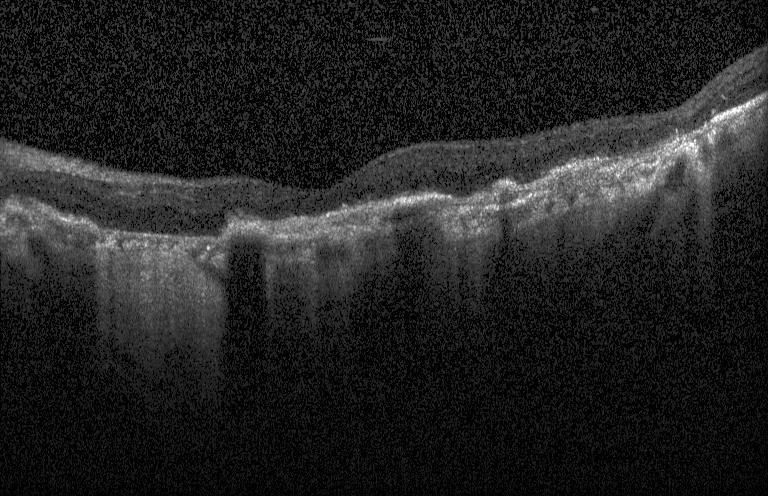

Macular scan · spectral-domain OCT · optical coherence tomography B-scan · Heidelberg Spectralis OCT system. Macular OCT: choroidal neovascularization (CNV).